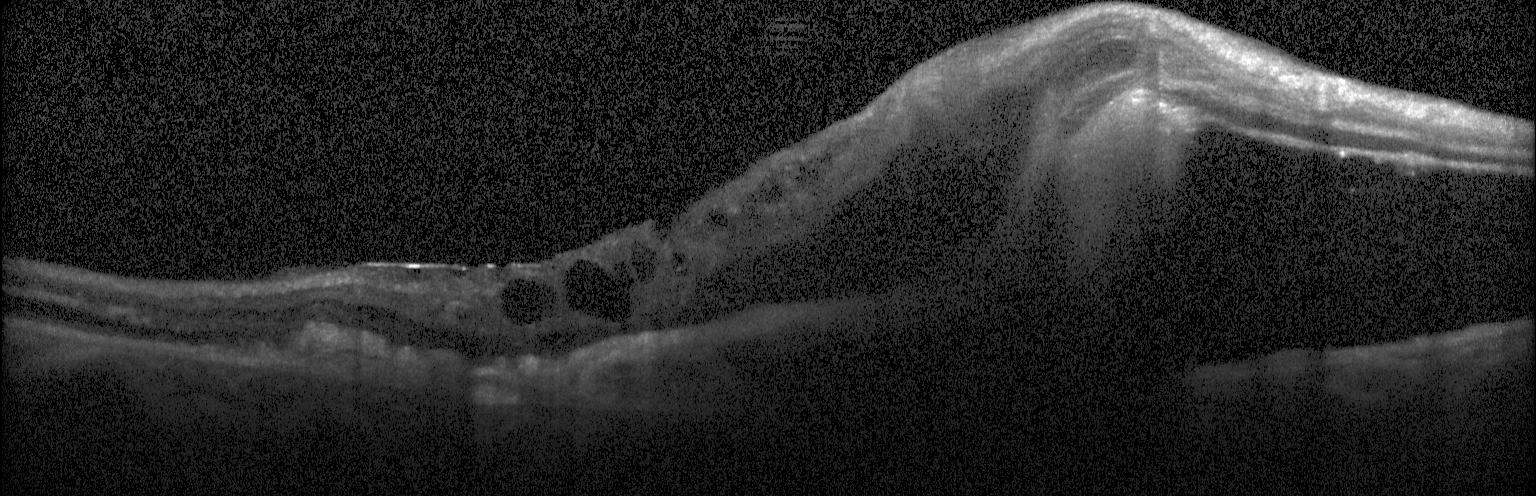

Dx: choroidal neovascularization.